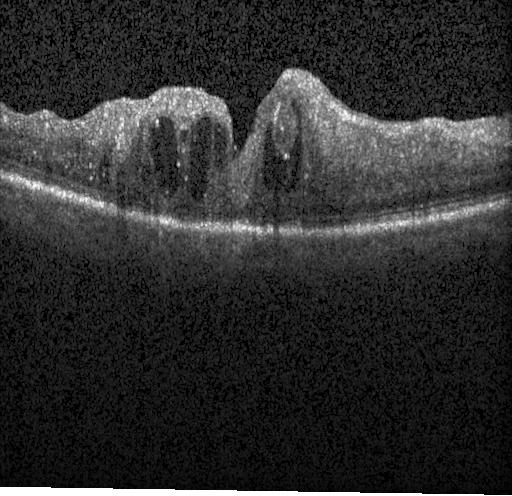 Spectral-domain optical coherence tomography · optical coherence tomography B-scan. Dx: diabetic macular edema (DME).